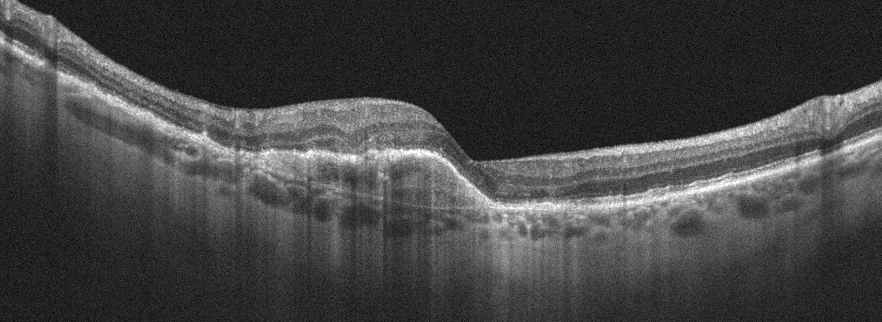
OS. Optical coherence tomography scan.
Assessment: AMD.